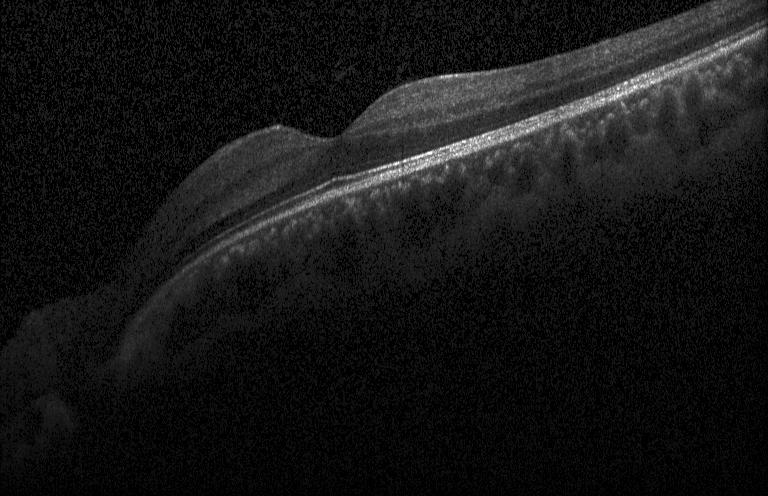 Macular OCT: no choroidal neovascularization, no diabetic macular edema, and no drusen.